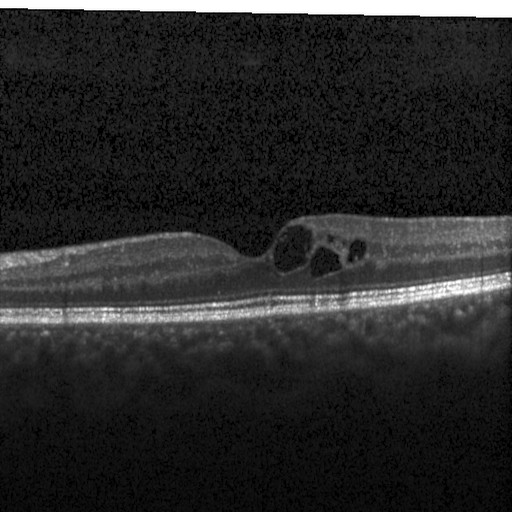
Retinal OCT cross-section showing diabetic macular edema (DME).